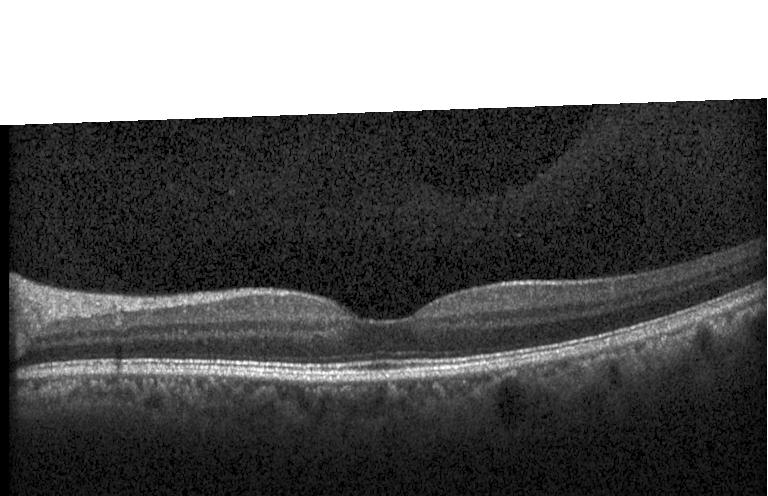
Heidelberg Spectralis OCT system; optical coherence tomography scan; spectral-domain optical coherence tomography
Finding: no evidence of choroidal neovascularization, diabetic macular edema, or drusen.